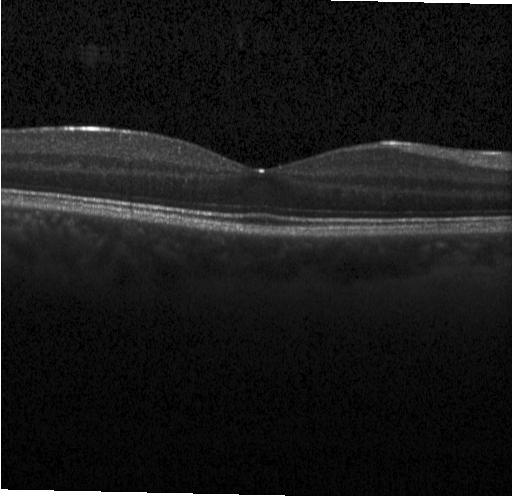 Macular OCT demonstrating no evidence of choroidal neovascularization, diabetic macular edema, or drusen.